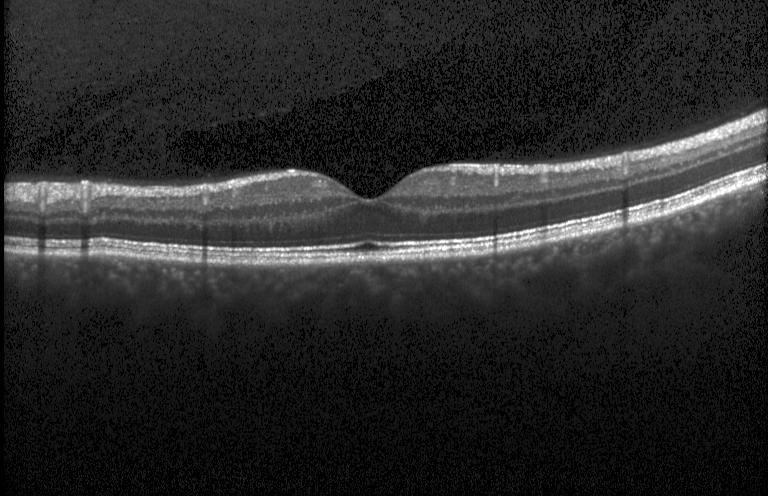

Macular OCT demonstrating no evidence of choroidal neovascularization, diabetic macular edema, or drusen.